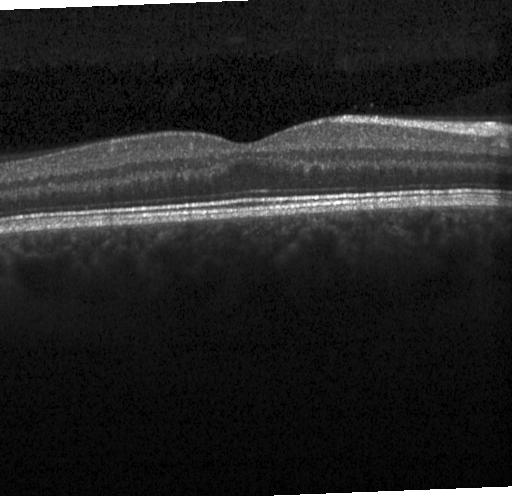

Through the macula · optical coherence tomography scan · spectral-domain optical coherence tomography · Heidelberg Spectralis.
Diagnosis: no CNV, no DME, and no drusen.